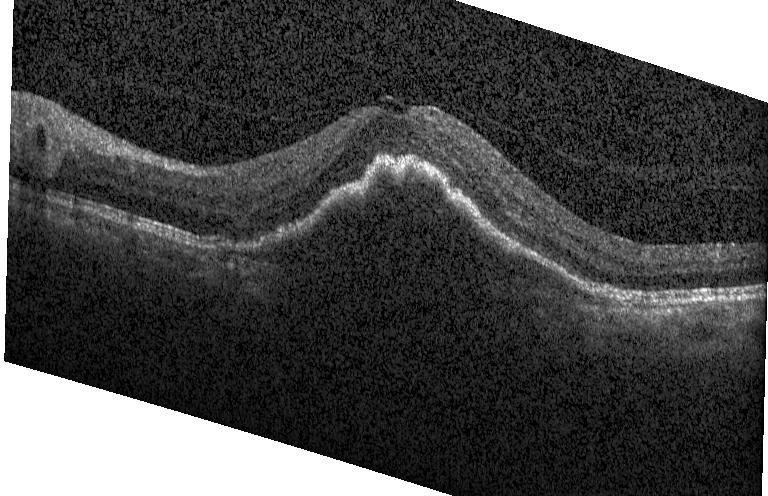 Finding: choroidal neovascularization.